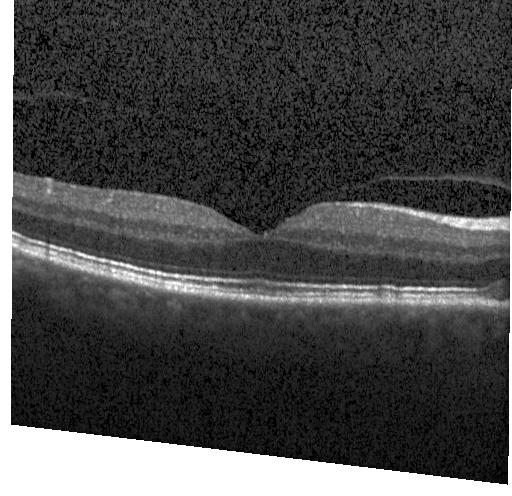
Finding: no evidence of choroidal neovascularization, diabetic macular edema, or drusen.